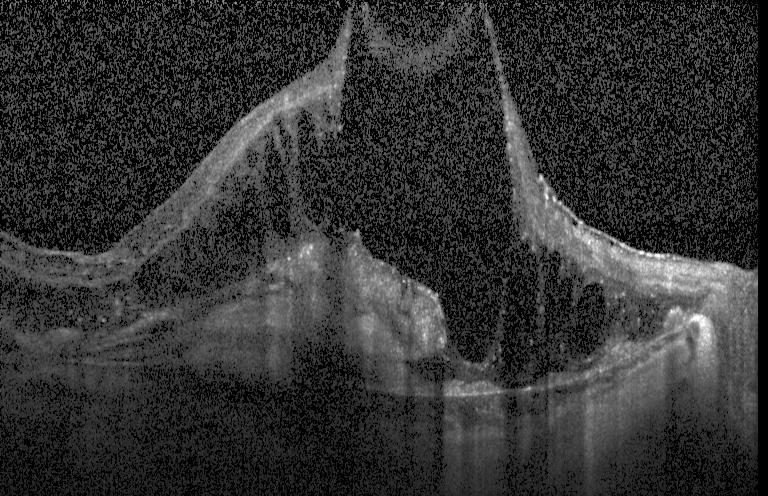

Centered on the fovea. Spectral-domain OCT. Heidelberg Spectralis OCT system. OCT B-scan
Finding: a choroidal neovascular membrane.